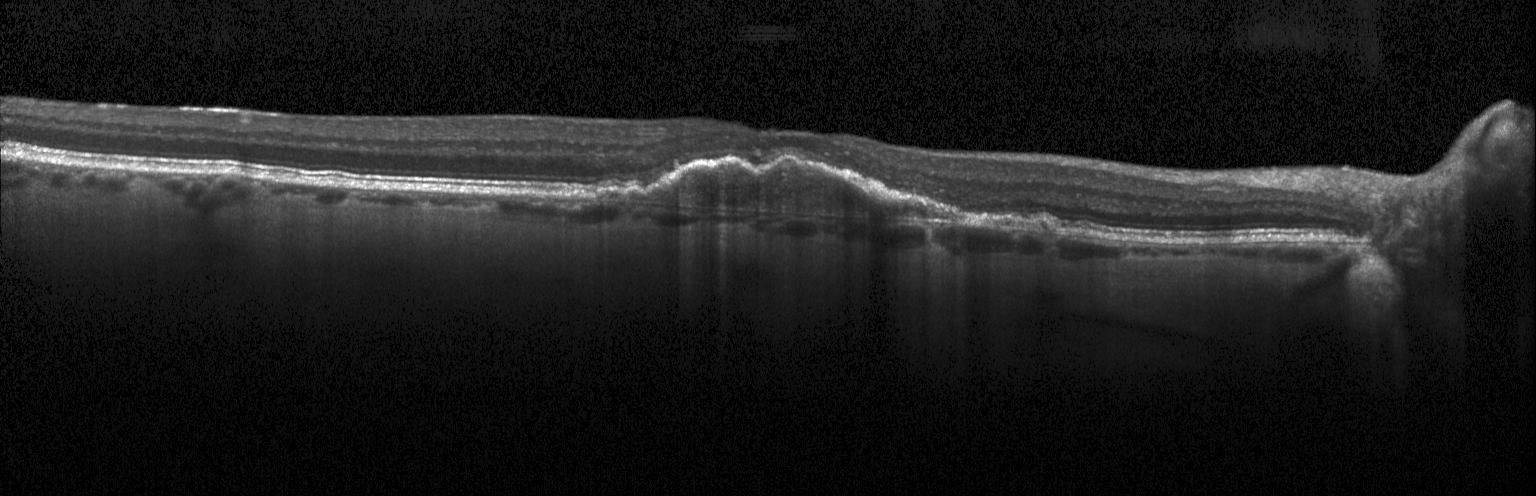 Macular OCT: choroidal neovascularization (CNV).